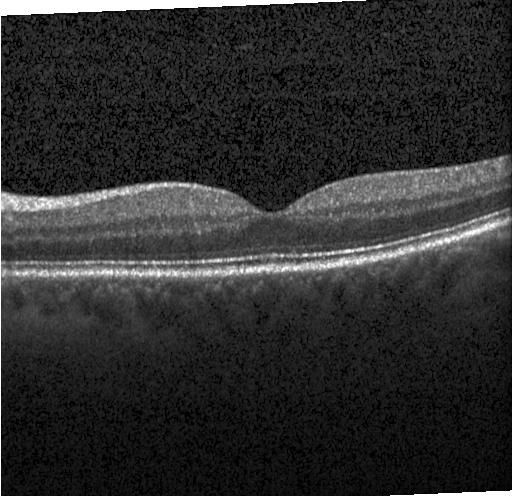

SD-OCT, OCT line scan, Heidelberg Spectralis OCT system — Diagnosis: no CNV, DME, or drusen.